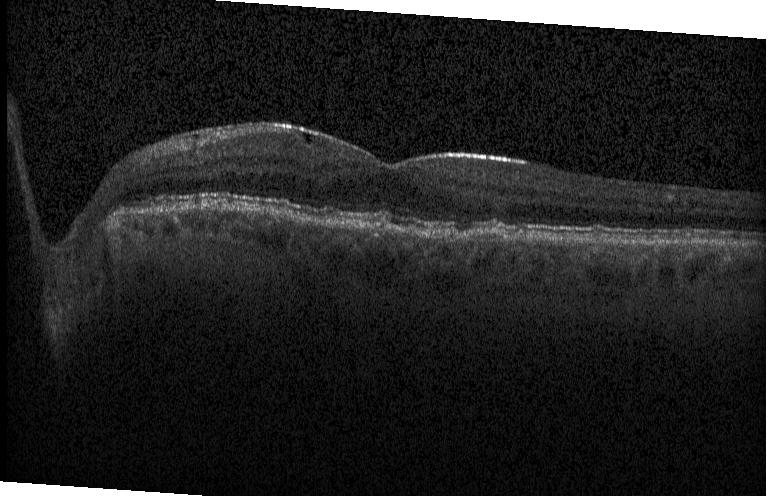

Retinal OCT B-scan
Finding: sub-RPE drusenoid deposits.